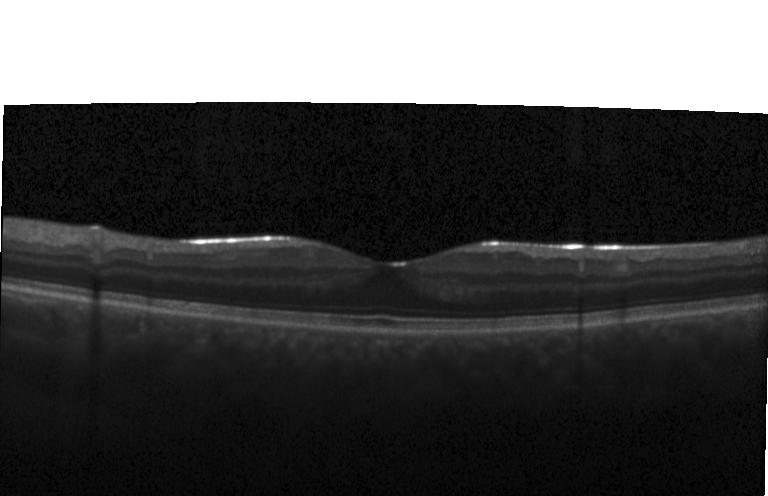 No CNV, DME, or drusen.